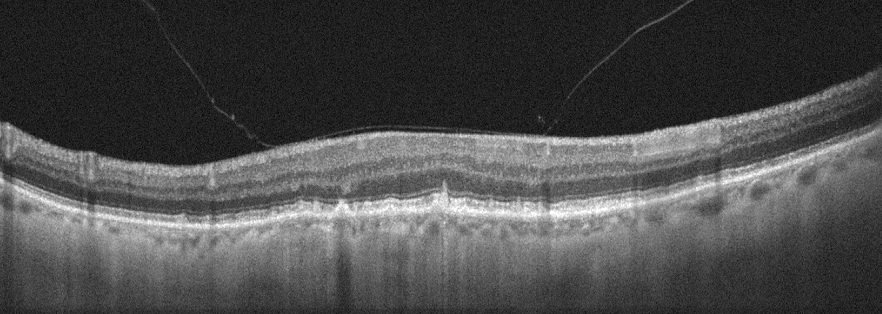
Acquired on an Optovue Avanti RTVue XR. OCT line scan. Oculus dexter. Through the macula — This B-scan demonstrates AMD.